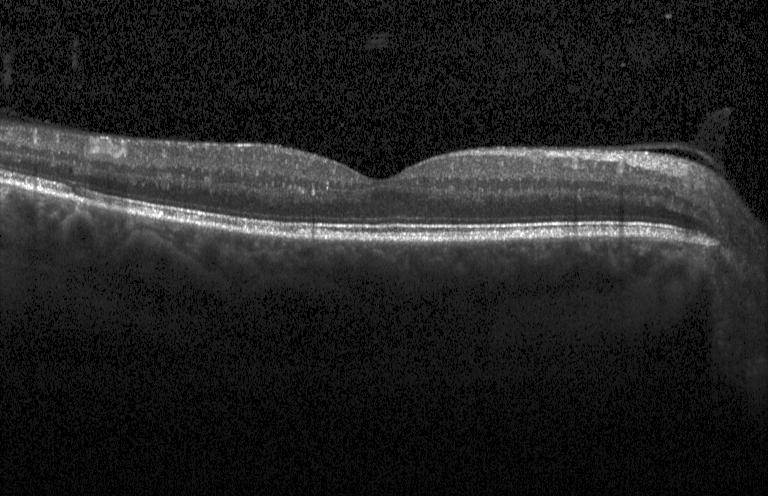 Through the macula, spectral-domain OCT, optical coherence tomography B-scan.
Dx: no choroidal neovascularization, no diabetic macular edema, and no drusen.